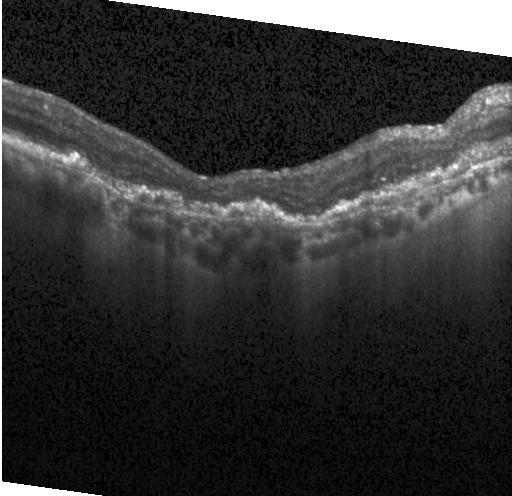
OCT finding: choroidal neovascularization.